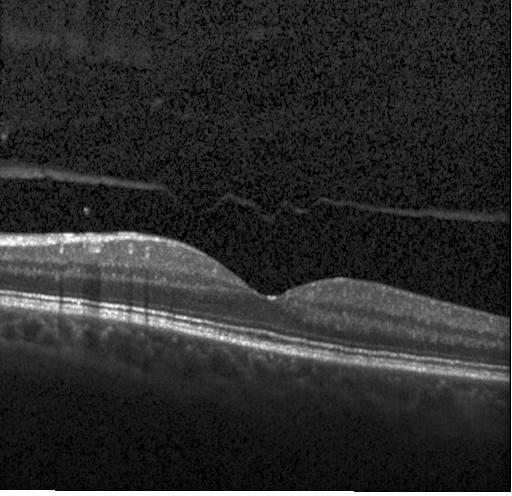
Acquired on a Heidelberg Spectralis · optical coherence tomography scan. This B-scan demonstrates neither choroidal neovascularization, diabetic macular edema, nor drusen.